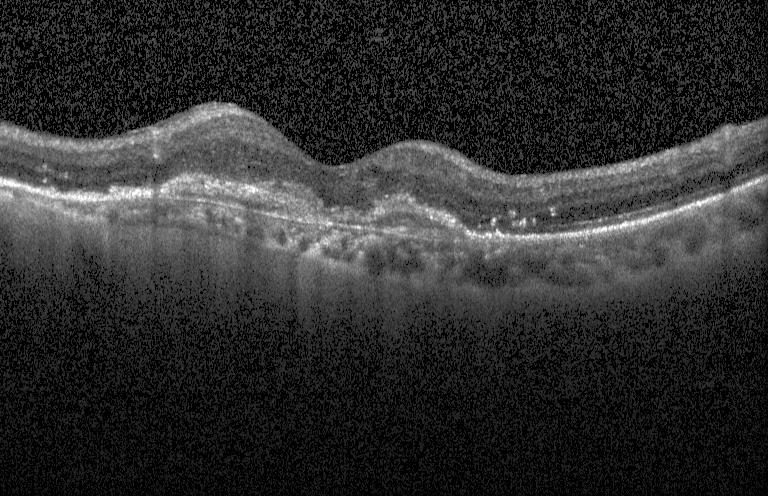

Acquired on a Heidelberg Spectralis, OCT B-scan, spectral-domain optical coherence tomography
Impression: CNV.